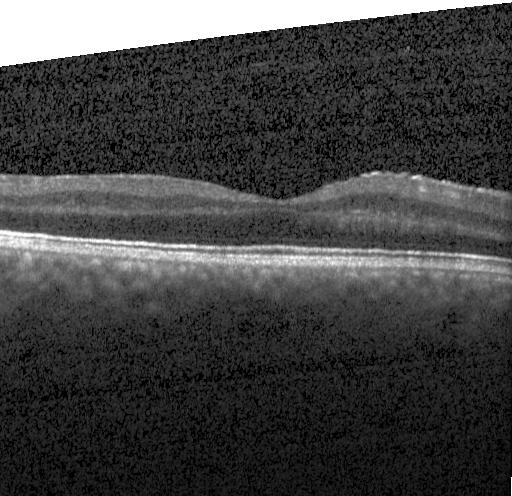
OCT B-scan — Impression: DME.